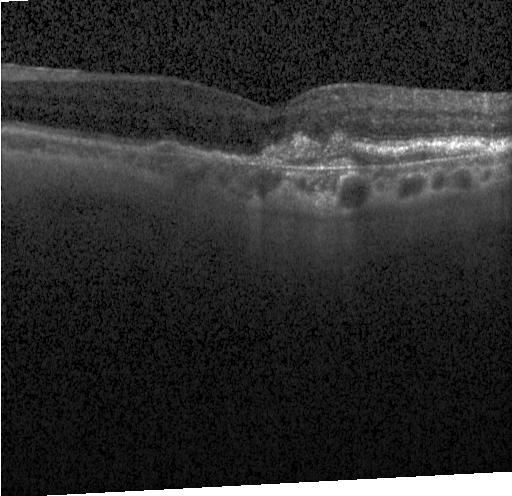
Retinal OCT cross-section, centered on the fovea — Finding: CNV.